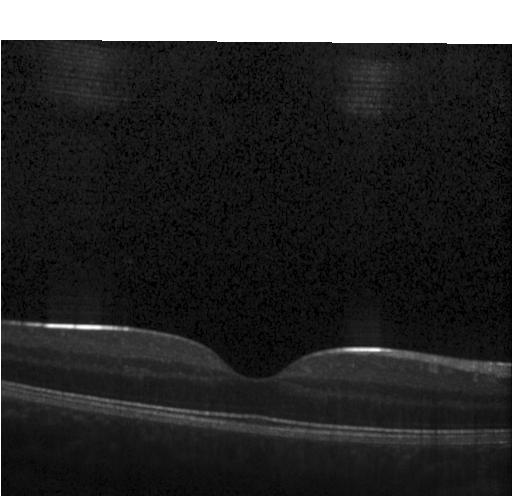
OCT finding: no choroidal neovascularization, diabetic macular edema, or drusen.